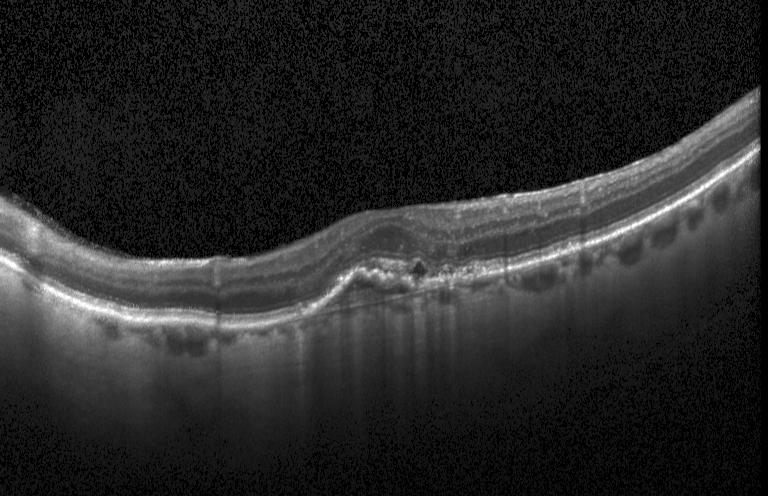 Retinal OCT cross-section
OCT finding: choroidal neovascularization (CNV).